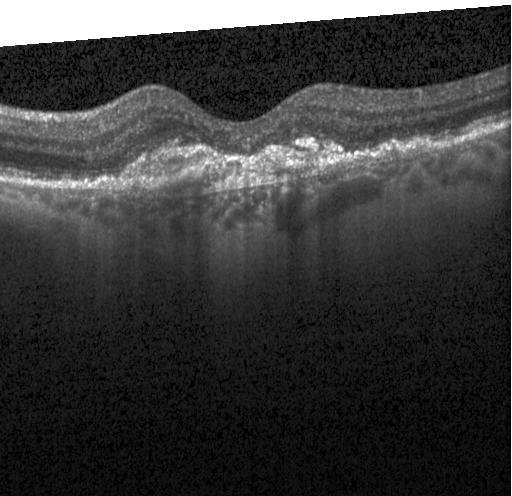
Dx: CNV.